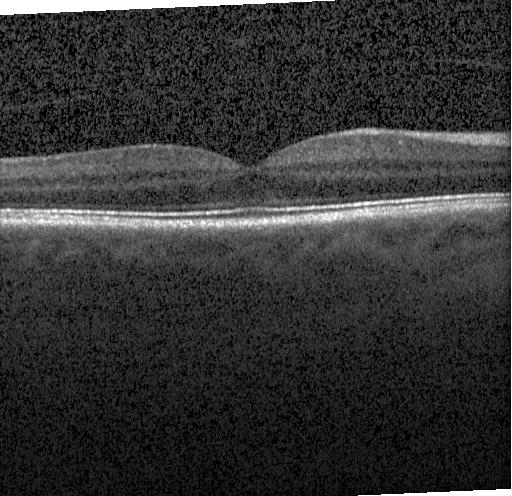 Centered on the fovea, retinal OCT B-scan, Heidelberg Spectralis
Finding: no choroidal neovascularization, diabetic macular edema, or drusen.